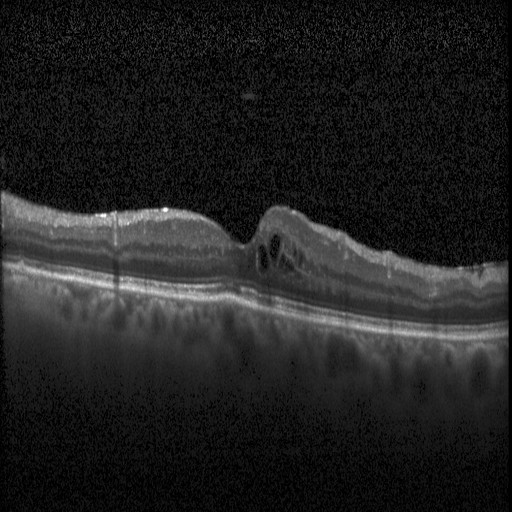
Retinal OCT B-scan.
This B-scan demonstrates DME.